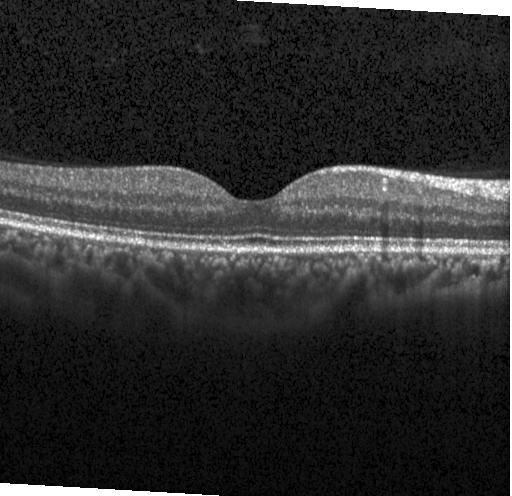
Dx: no choroidal neovascularization, diabetic macular edema, or drusen.